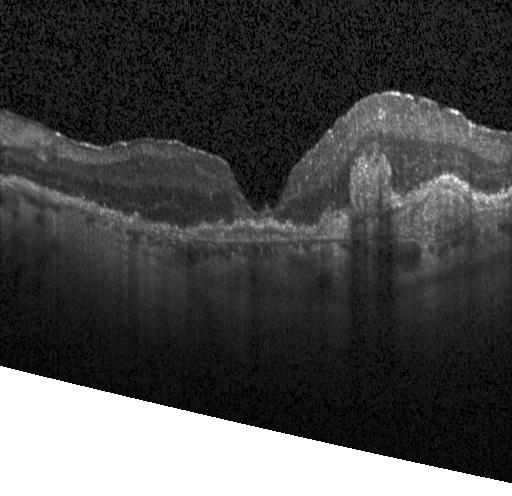 Fovea-centered, spectral-domain optical coherence tomography, instrument: Heidelberg Spectralis, optical coherence tomography scan.
Diagnosis: choroidal neovascularization (CNV).